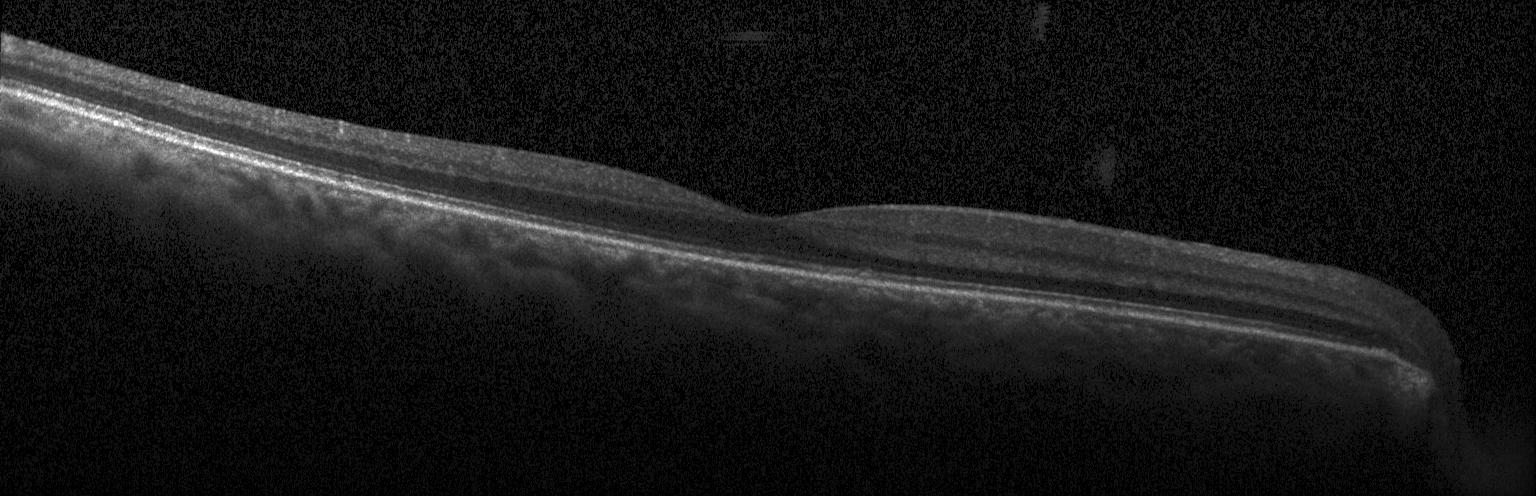 This B-scan demonstrates no choroidal neovascularization, diabetic macular edema, or drusen.